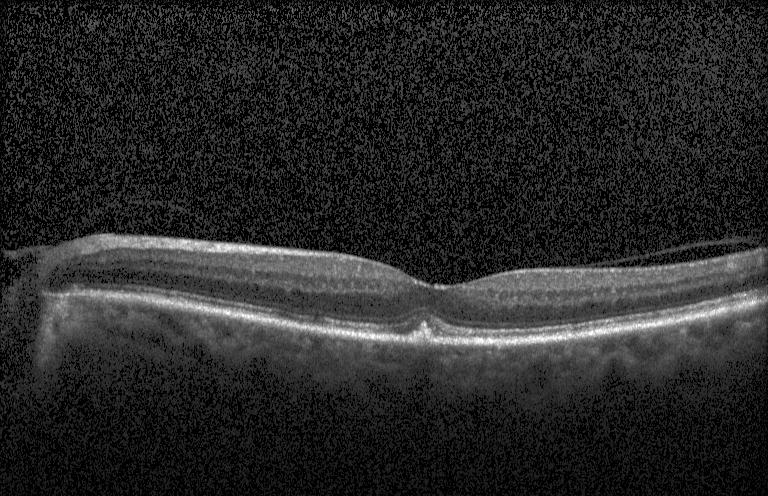

Diagnosis: multiple drusen.